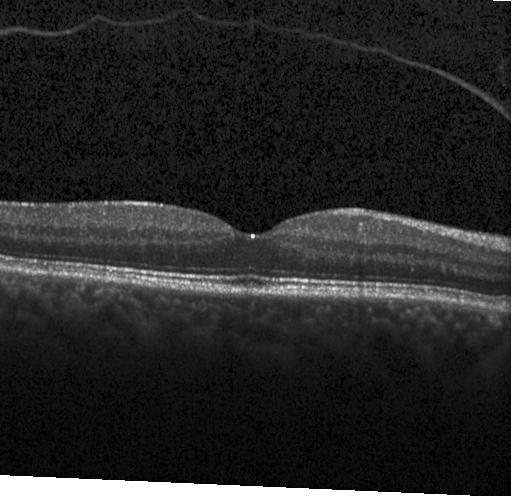 No choroidal neovascularization, diabetic macular edema, or drusen.